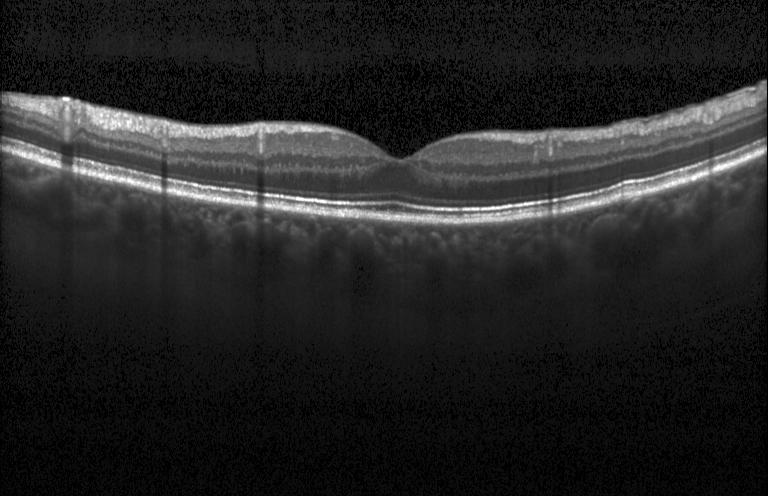
No evidence of choroidal neovascularization, diabetic macular edema, or drusen.